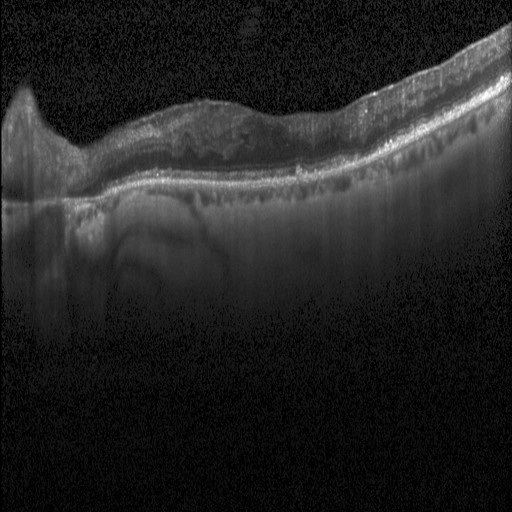 OCT scan showing diabetic macular edema (DME).